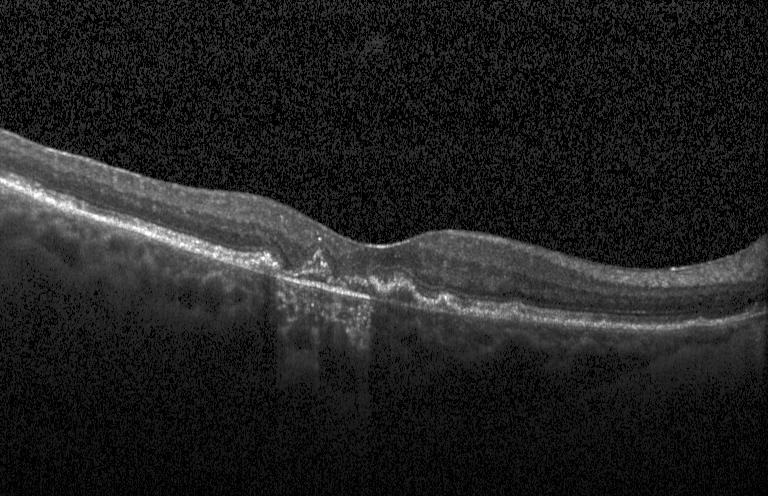 Spectral-domain optical coherence tomography, through the macula, OCT B-scan, Heidelberg Spectralis OCT system.
Finding: a choroidal neovascular membrane.